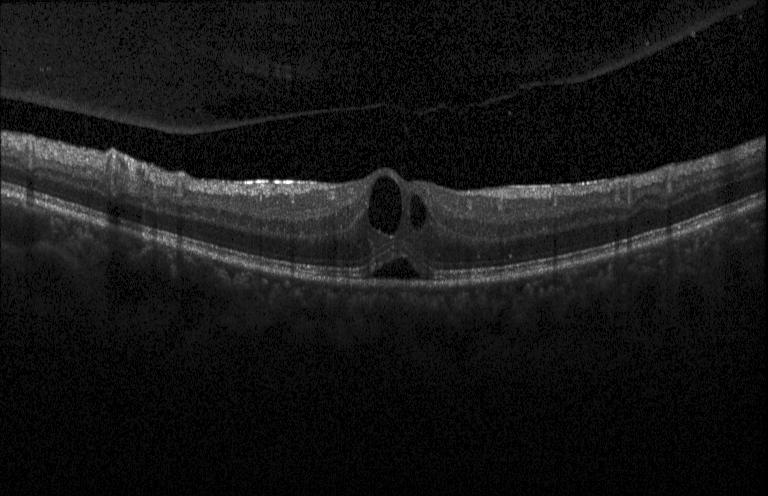

Impression: DME.